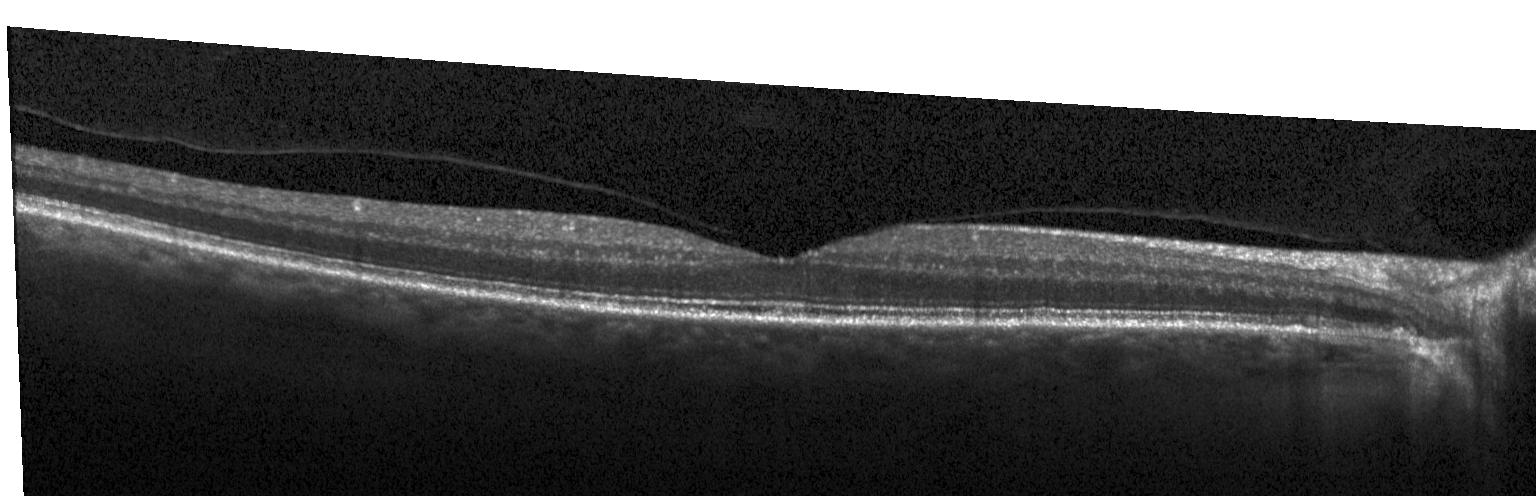
Optical coherence tomography scan — Dx: no choroidal neovascularization, no diabetic macular edema, and no drusen.